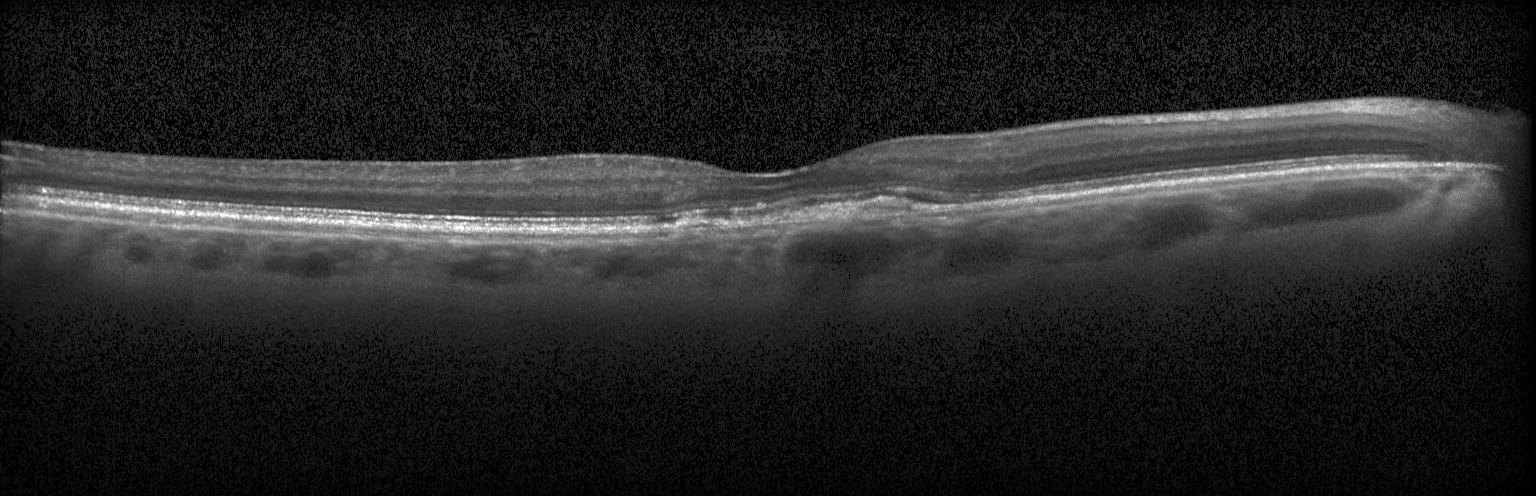 Dx: CNV.